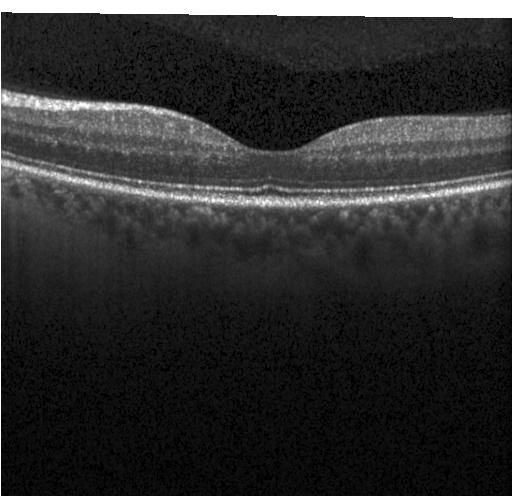 OCT line scan, spectral-domain optical coherence tomography, centered on the fovea. The scan shows no CNV, no DME, and no drusen.